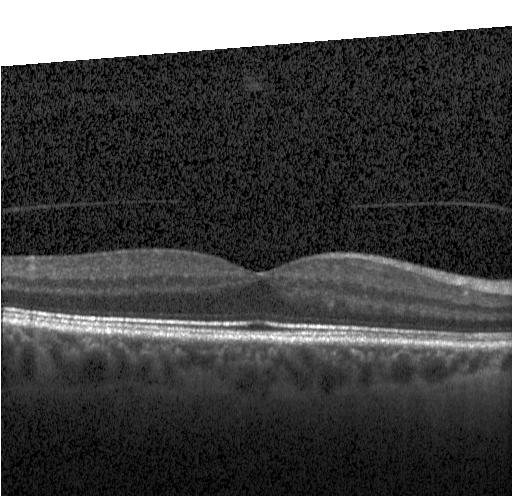
Retinal OCT cross-section, acquired on a Heidelberg Spectralis, spectral-domain OCT
Finding: no CNV, no DME, and no drusen.